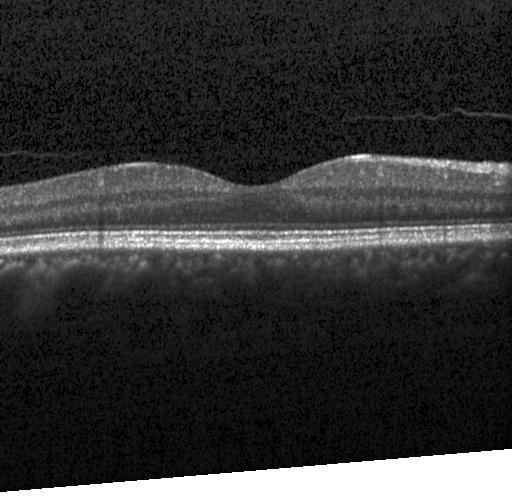 OCT B-scan. Finding: neither choroidal neovascularization, diabetic macular edema, nor drusen.